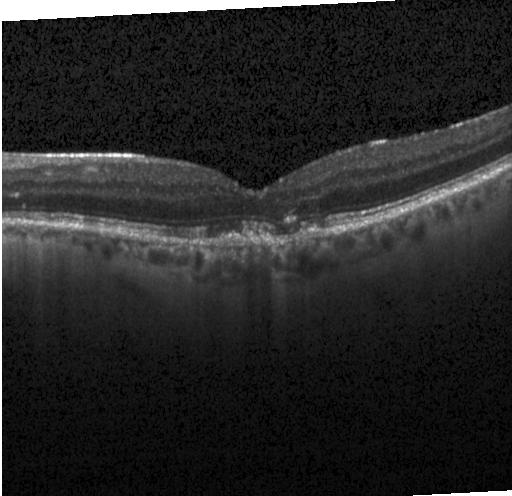 Retinal OCT B-scan. Macular scan. Instrument: Heidelberg Spectralis. Spectral-domain OCT.
Impression: choroidal neovascularization (CNV).